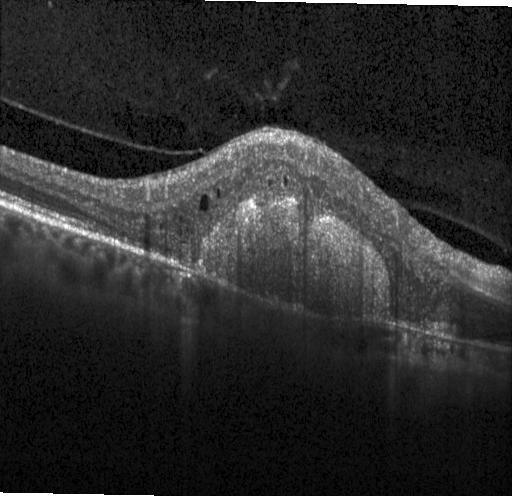 OCT finding: choroidal neovascularization (CNV).